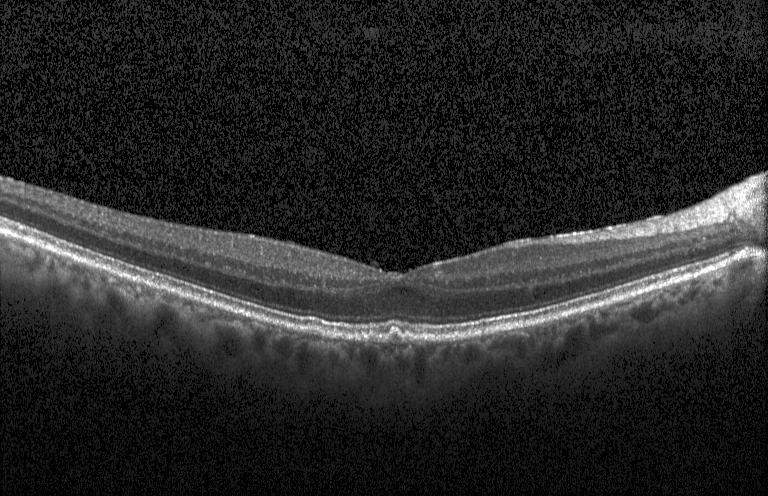
Retinal OCT B-scan · instrument: Heidelberg Spectralis · spectral-domain optical coherence tomography · centered on the fovea. Dx: drusen.